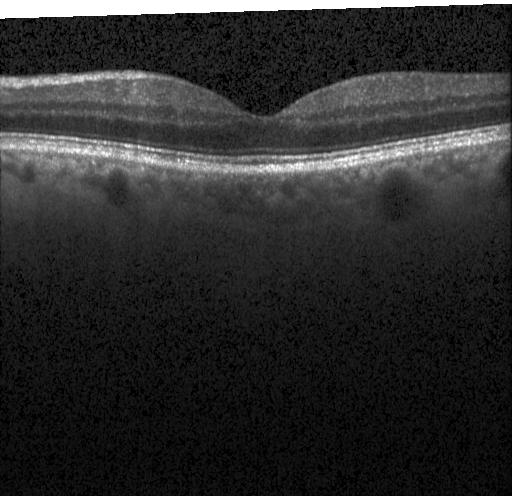
Finding: neither CNV, DME, nor drusen.